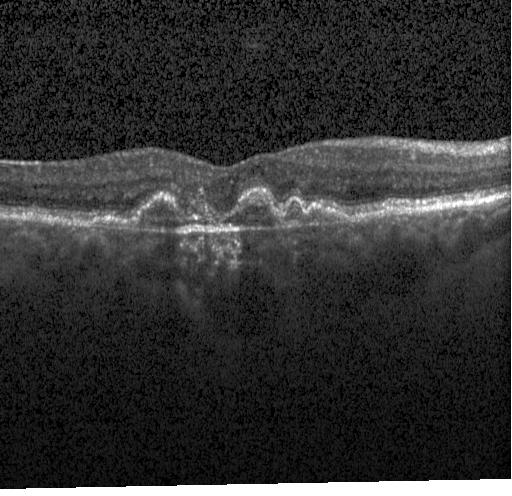
Assessment: a choroidal neovascular membrane.